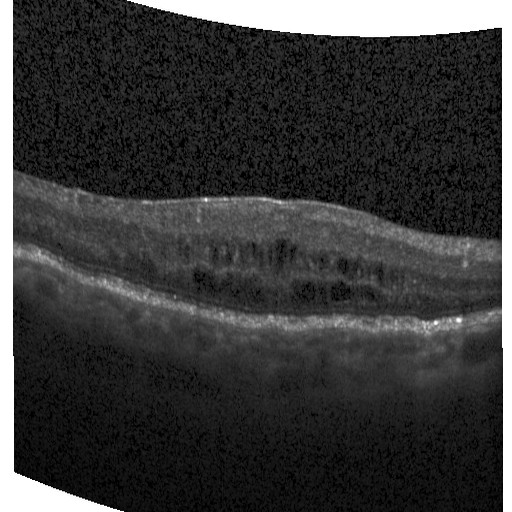 Macular OCT demonstrating DME.